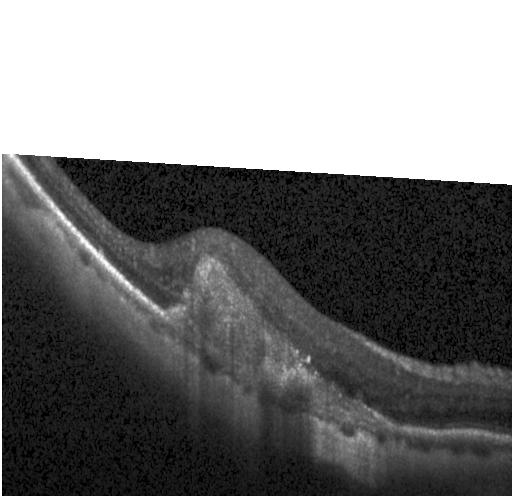
OCT B-scan.
The scan shows choroidal neovascularization.